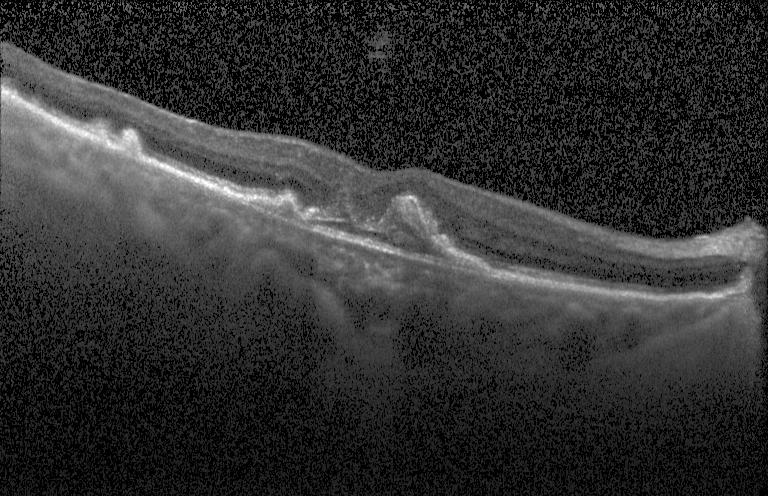
Finding: choroidal neovascularization.